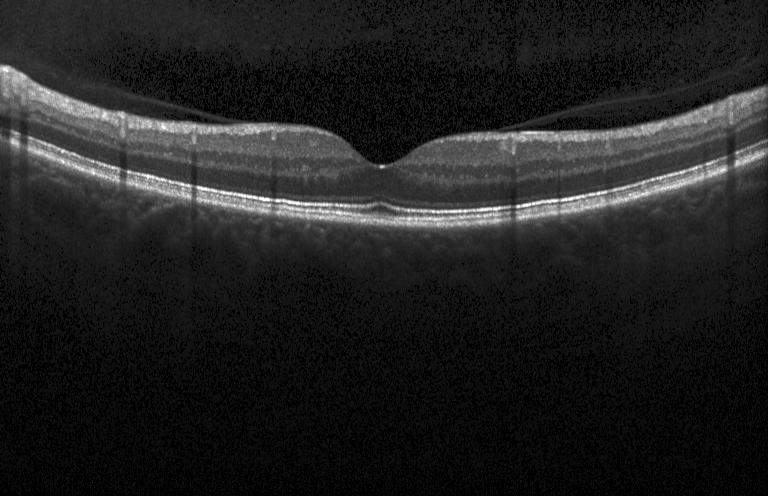 This B-scan demonstrates no evidence of choroidal neovascularization, diabetic macular edema, or drusen.